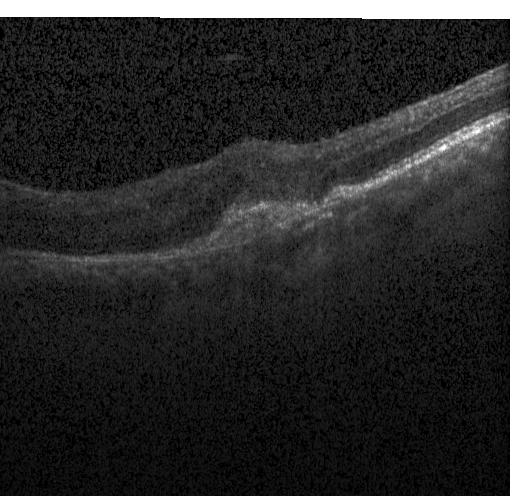
Retinal OCT B-scan, spectral-domain OCT, Heidelberg Spectralis OCT system
The scan shows a choroidal neovascular membrane.